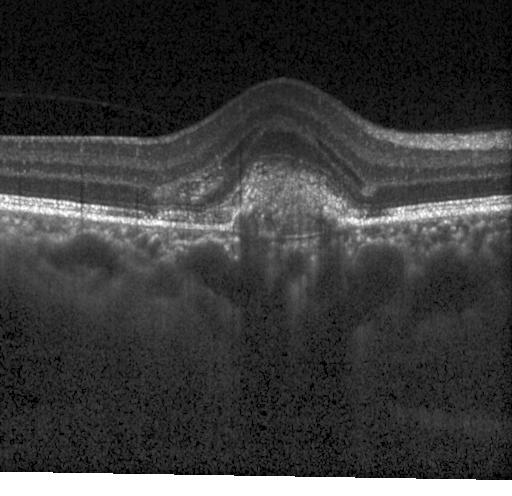 Heidelberg Spectralis, optical coherence tomography scan.
Impression: a choroidal neovascular membrane.